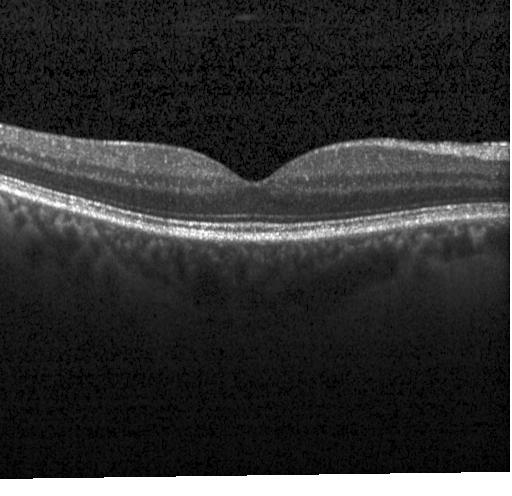

Heidelberg Spectralis OCT system · OCT B-scan — No CNV, no DME, and no drusen.